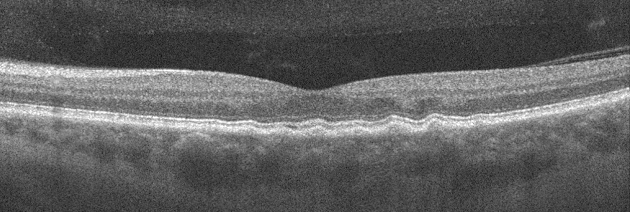 Oculus sinister · instrument: Optovue Avanti RTVue XR · optical coherence tomography B-scan.
OCT finding: age-related macular degeneration.